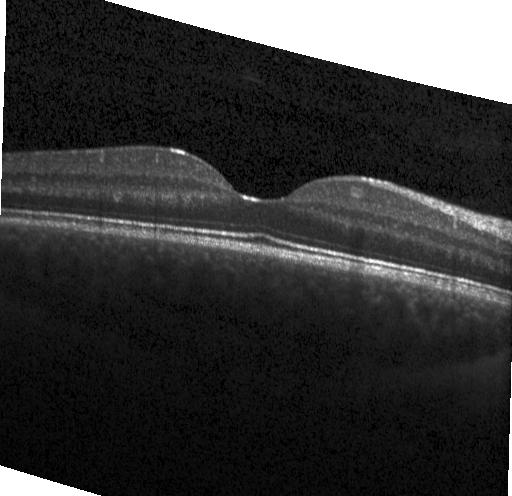
Retinal OCT B-scan
Impression: neither choroidal neovascularization, diabetic macular edema, nor drusen.